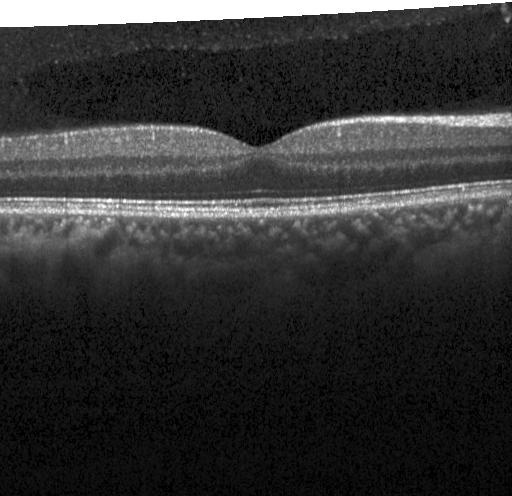

Retinal OCT B-scan · acquired on a Heidelberg Spectralis — No evidence of choroidal neovascularization, diabetic macular edema, or drusen.